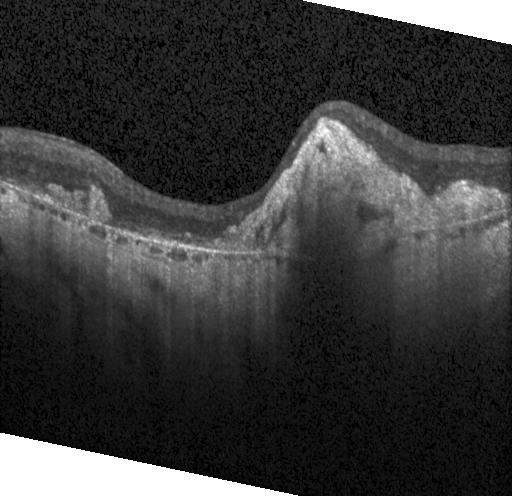

Finding: a choroidal neovascular membrane.